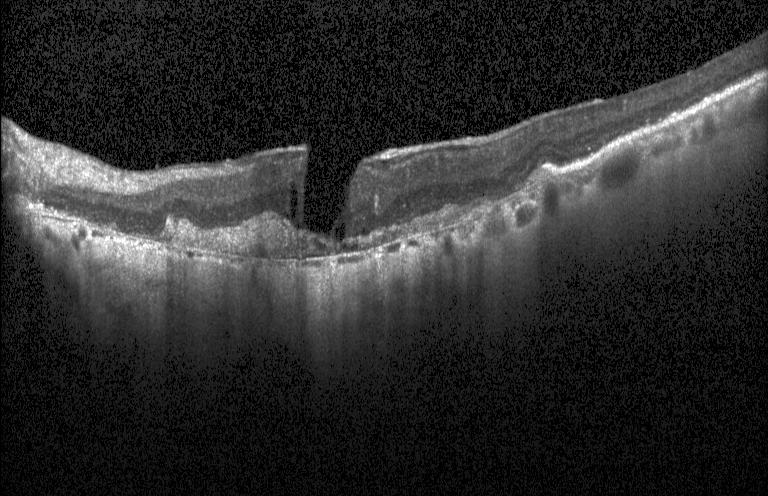

SD-OCT. Centered on the fovea. Optical coherence tomography scan — Impression: choroidal neovascularization (CNV).